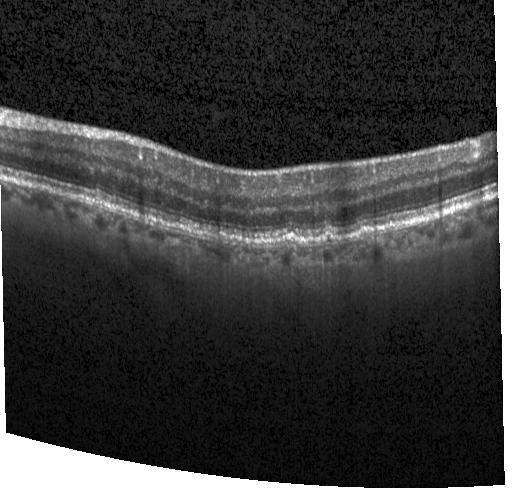 OCT B-scan — Finding: sub-RPE drusenoid deposits.